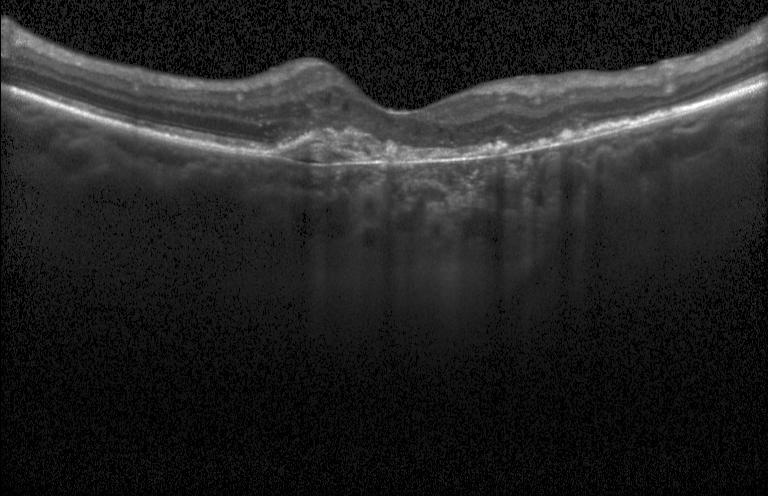

Optical coherence tomography scan. Spectral-domain OCT. Centered on the fovea — Diagnosis: CNV.